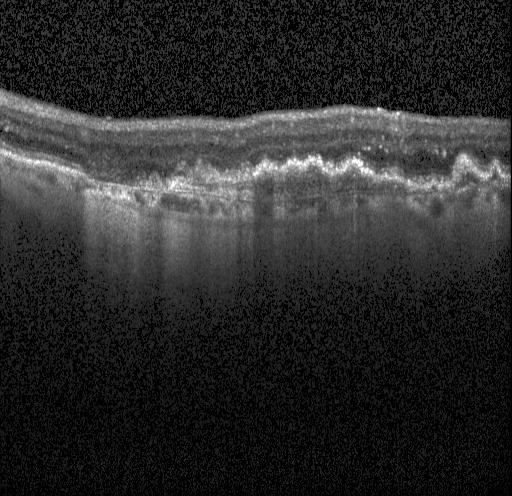
Retinal OCT cross-section
Finding: choroidal neovascularization.